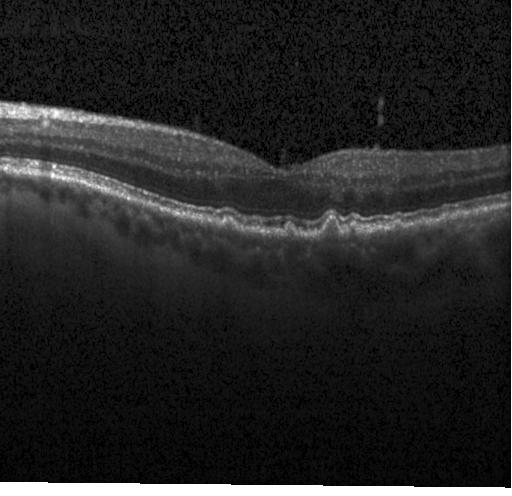 Dx: multiple drusen.